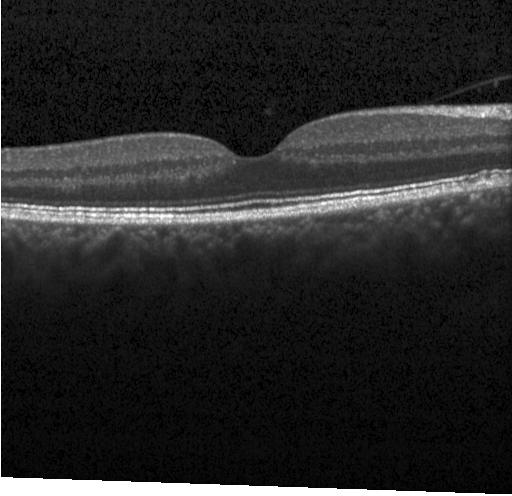
Optical coherence tomography B-scan; spectral-domain OCT. The scan shows neither choroidal neovascularization, diabetic macular edema, nor drusen.